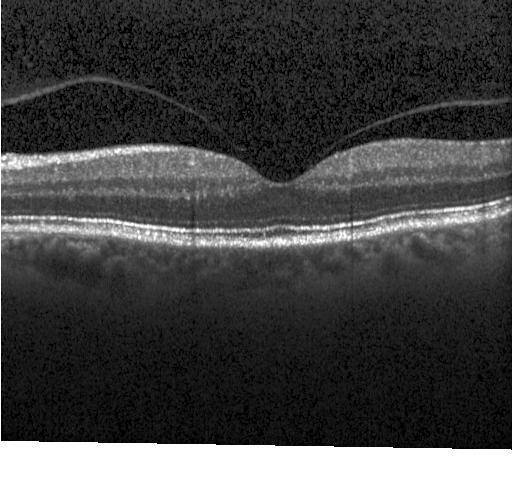 OCT B-scan — Impression: no choroidal neovascularization, no diabetic macular edema, and no drusen.